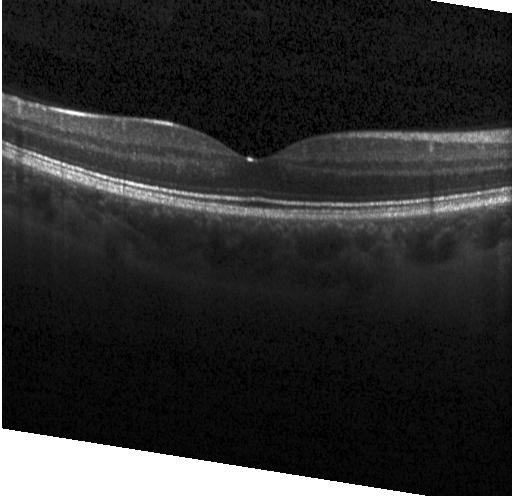 OCT finding: no choroidal neovascularization, diabetic macular edema, or drusen.